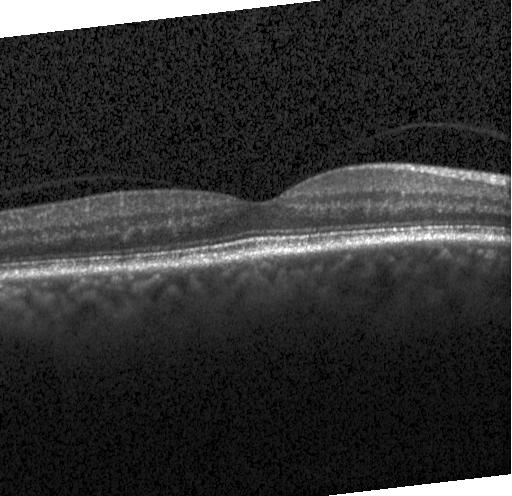 Fovea-centered, SD-OCT, retinal OCT cross-section, Heidelberg Spectralis OCT system
Finding: no evidence of choroidal neovascularization, diabetic macular edema, or drusen.